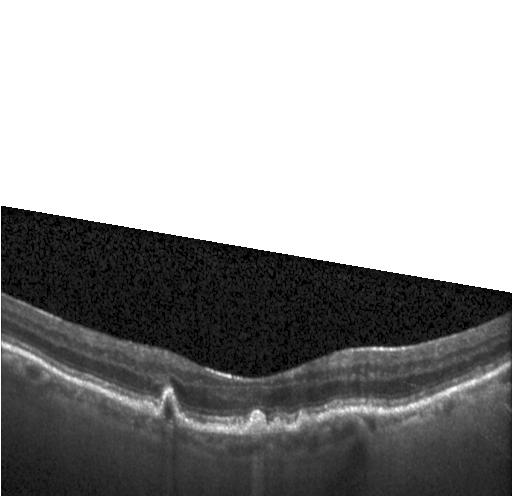

Diagnosis: sub-RPE drusenoid deposits.